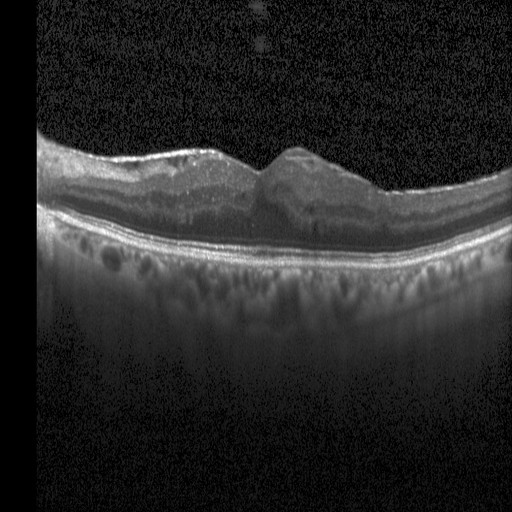

Optical coherence tomography scan, instrument: Heidelberg Spectralis — Diagnosis: diabetic macular edema.